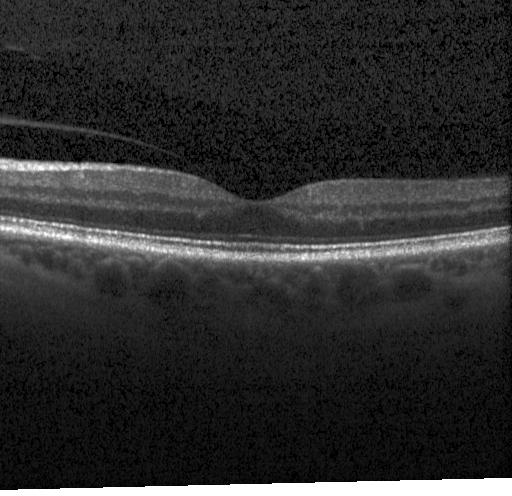 Diagnosis: no choroidal neovascularization, no diabetic macular edema, and no drusen.